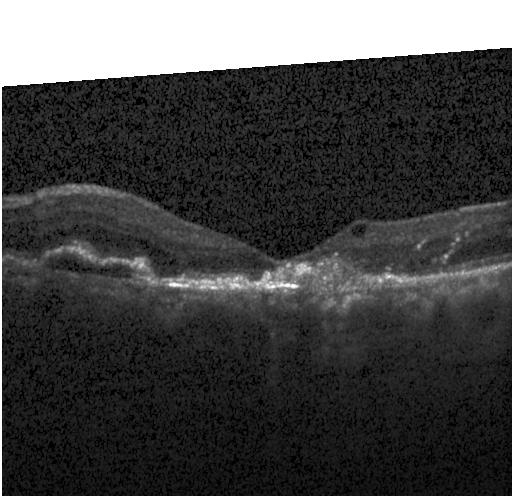 Optical coherence tomography scan, spectral-domain OCT. Diagnosis: a choroidal neovascular membrane.